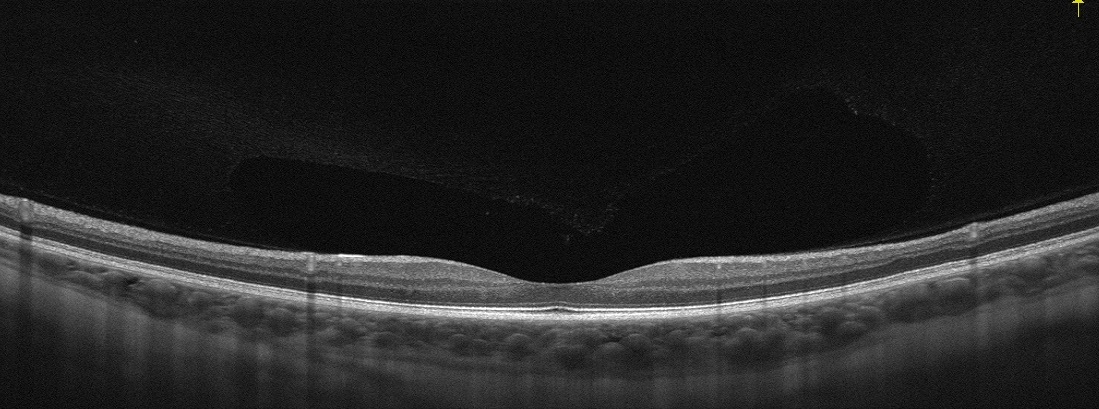
Through the macula. OCT line scan. Optovue Avanti RTVue XR. No AMD, DME, ERM, RAO, RVO, or VID.